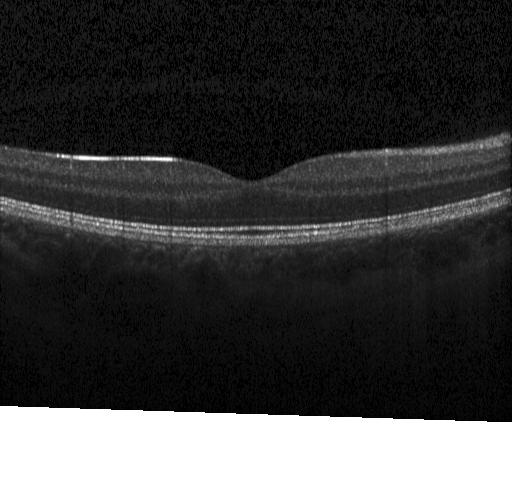

Impression: no choroidal neovascularization, diabetic macular edema, or drusen.